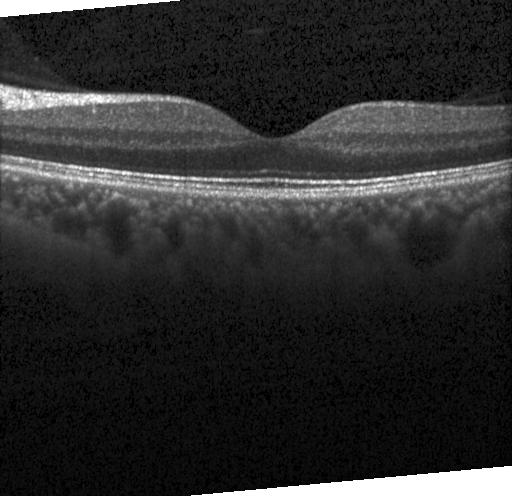

Macular OCT demonstrating no CNV, no DME, and no drusen.